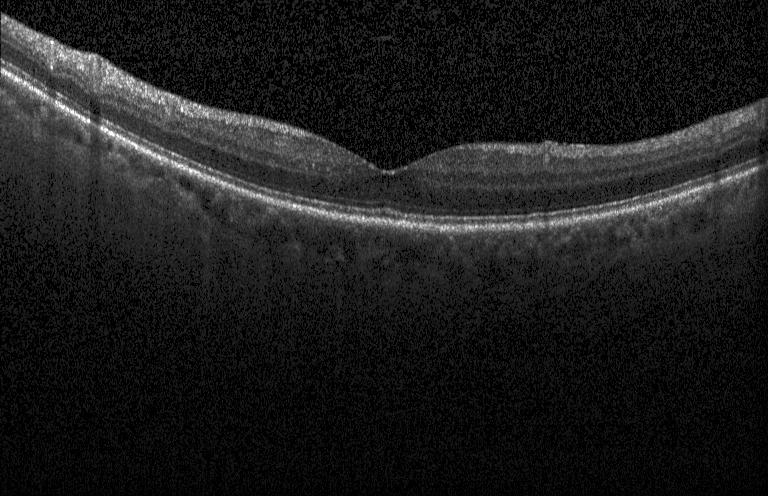

OCT line scan; horizontal scan through the fovea; spectral-domain optical coherence tomography. This B-scan demonstrates neither choroidal neovascularization, diabetic macular edema, nor drusen.